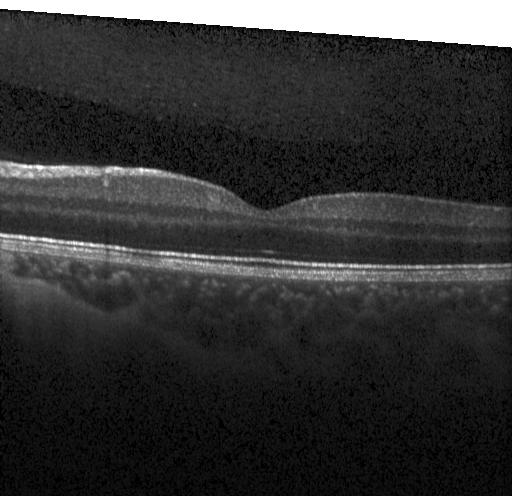
OCT line scan, horizontal scan through the fovea — Impression: no CNV, no DME, and no drusen.